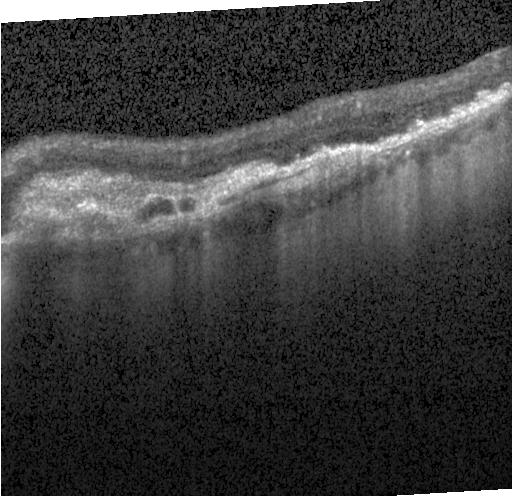 Assessment: a choroidal neovascular membrane.